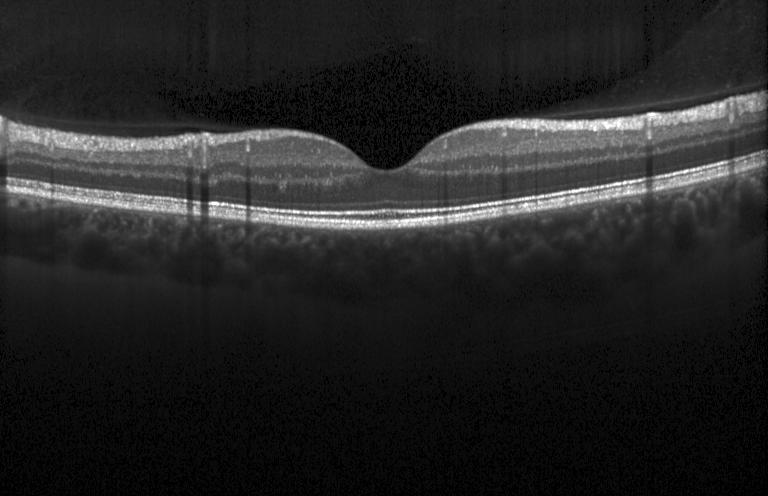

Acquired on a Heidelberg Spectralis, retinal OCT cross-section.
Diagnosis: no evidence of choroidal neovascularization, diabetic macular edema, or drusen.